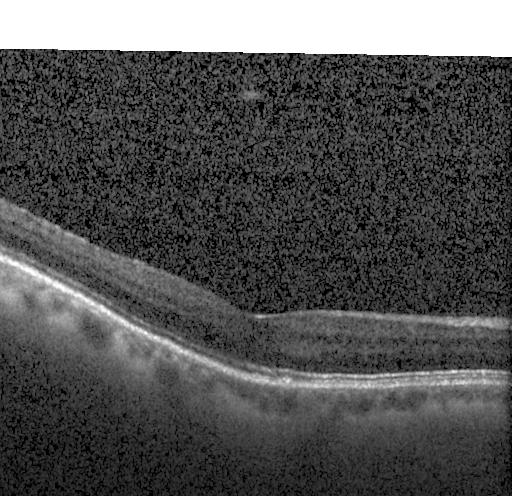 OCT B-scan. Finding: neither CNV, DME, nor drusen.